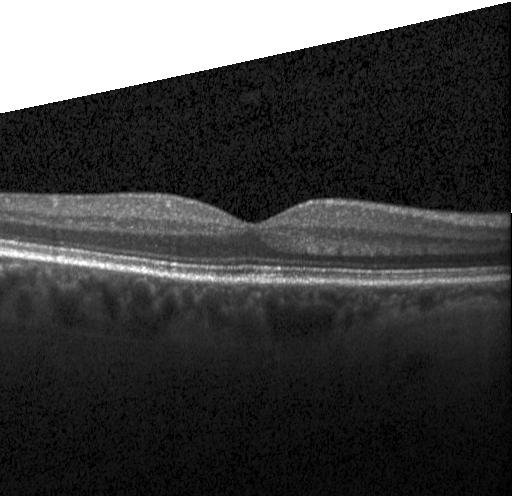
Dx: no choroidal neovascularization, diabetic macular edema, or drusen.